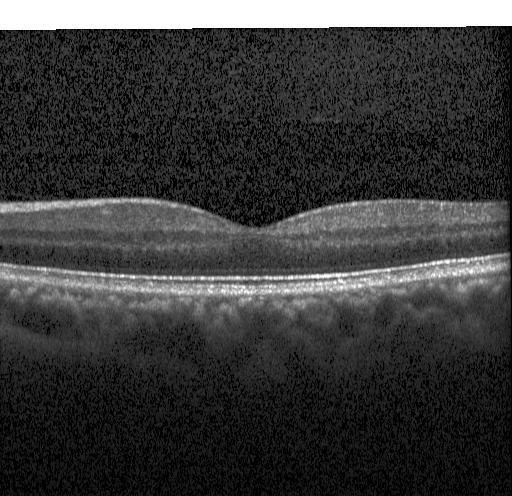 Retinal OCT cross-section. Heidelberg Spectralis OCT system. Spectral-domain optical coherence tomography
The scan shows no evidence of choroidal neovascularization, diabetic macular edema, or drusen.